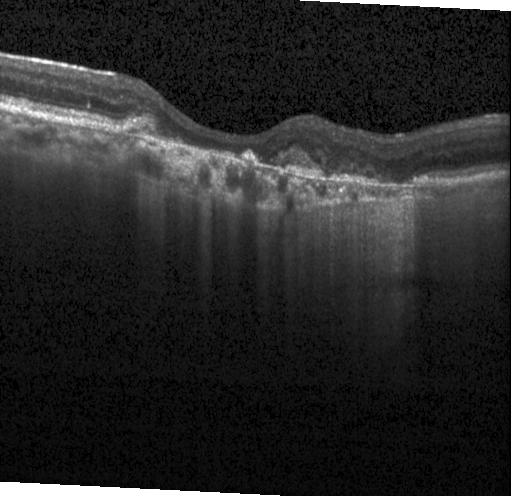

Instrument: Heidelberg Spectralis; SD-OCT; fovea-centered; OCT B-scan. The scan shows a choroidal neovascular membrane.